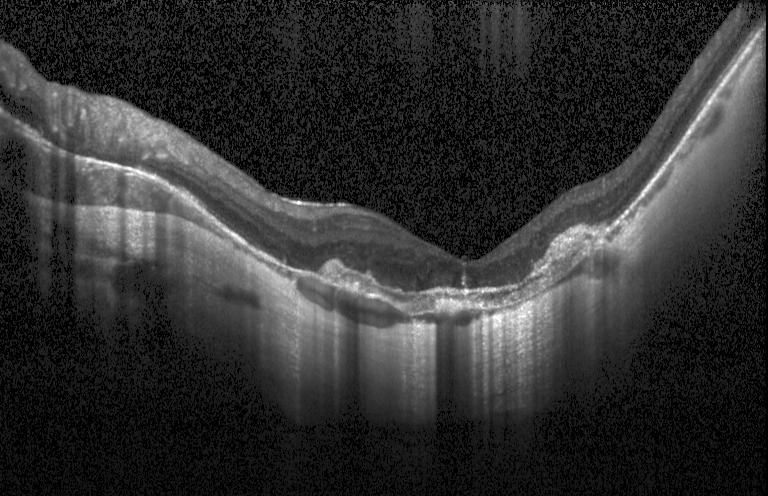
Spectral-domain OCT, fovea-centered, Heidelberg Spectralis, retinal OCT B-scan
OCT finding: choroidal neovascularization.